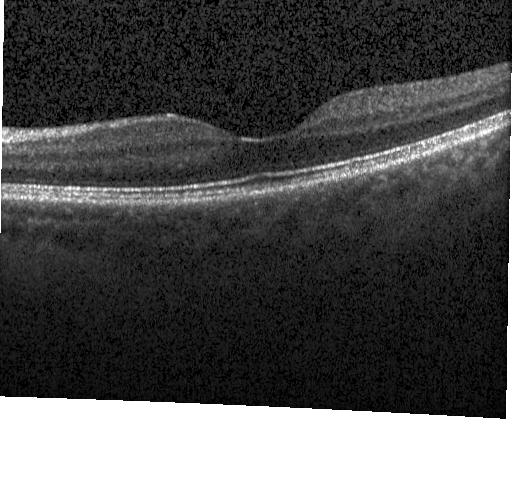 Macular scan, retinal OCT B-scan.
Impression: no choroidal neovascularization, diabetic macular edema, or drusen.